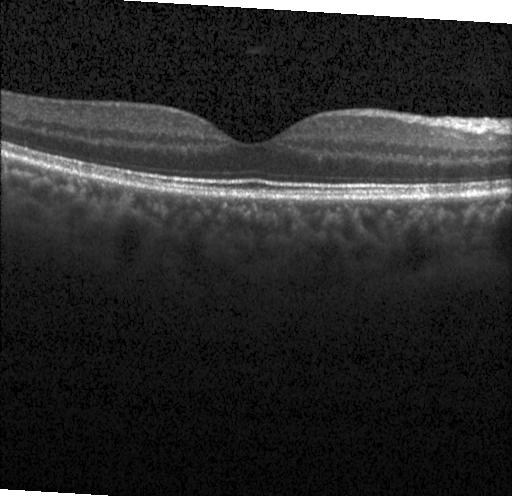

Acquired on a Heidelberg Spectralis; fovea-centered; retinal OCT B-scan — Diagnosis: no choroidal neovascularization, diabetic macular edema, or drusen.